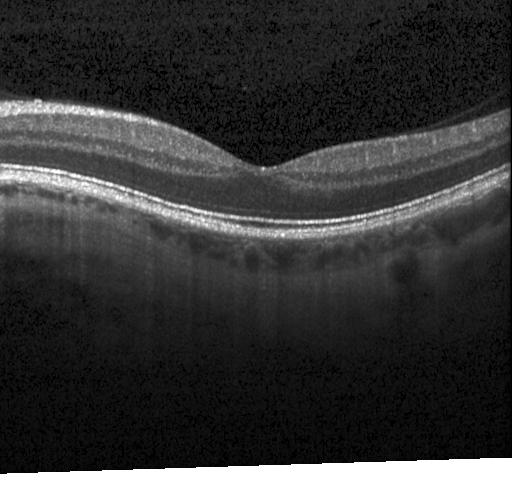
Spectral-domain OCT. Through the macula. Optical coherence tomography B-scan. Acquired on a Heidelberg Spectralis
Diagnosis: neither choroidal neovascularization, diabetic macular edema, nor drusen.